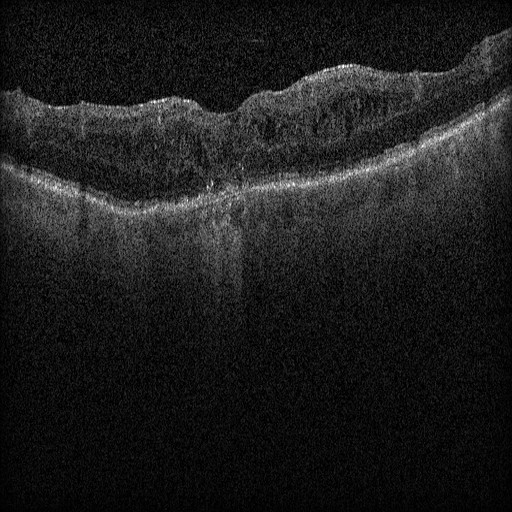

Optical coherence tomography B-scan — Diagnosis: DME.